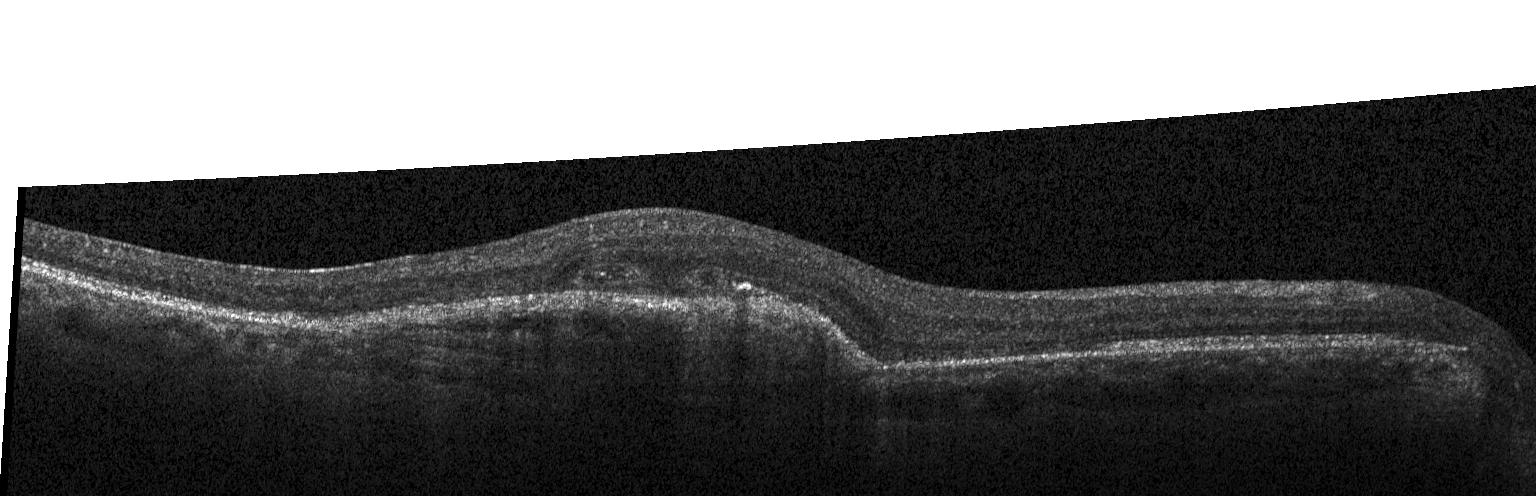 OCT B-scan — Assessment: a choroidal neovascular membrane.